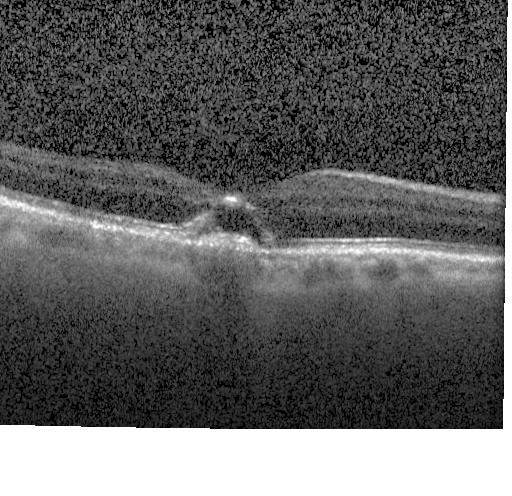 Optical coherence tomography scan.
Assessment: a choroidal neovascular membrane.